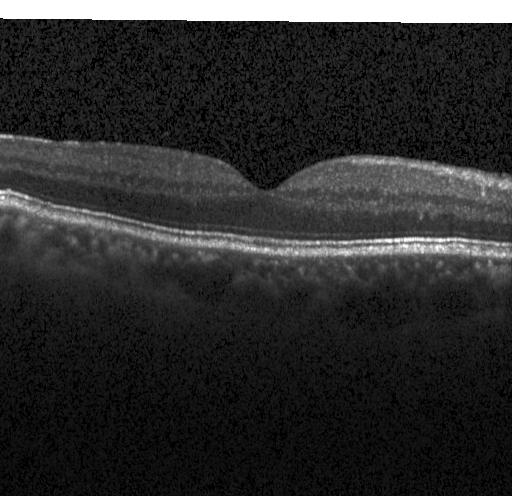 Heidelberg Spectralis. Optical coherence tomography B-scan. Finding: neither choroidal neovascularization, diabetic macular edema, nor drusen.